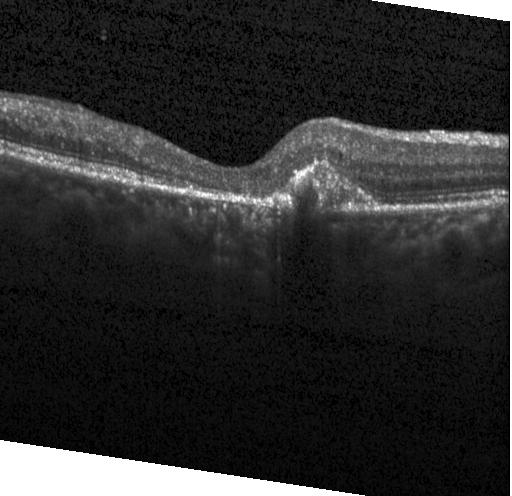 Optical coherence tomography scan.
Assessment: choroidal neovascularization (CNV).